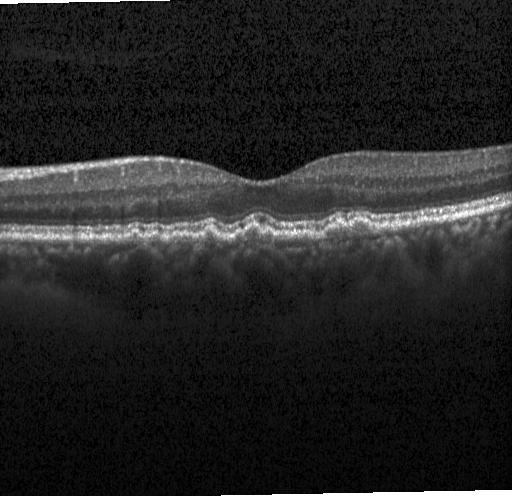 Drusen.